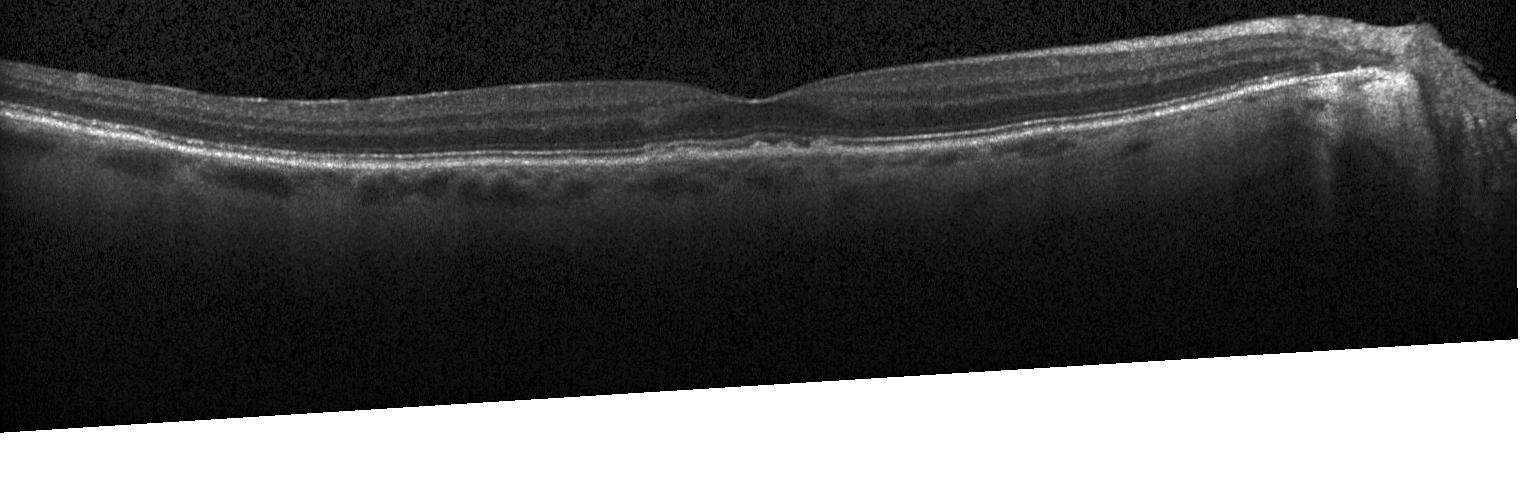 Retinal OCT cross-section; spectral-domain optical coherence tomography
Impression: multiple drusen.